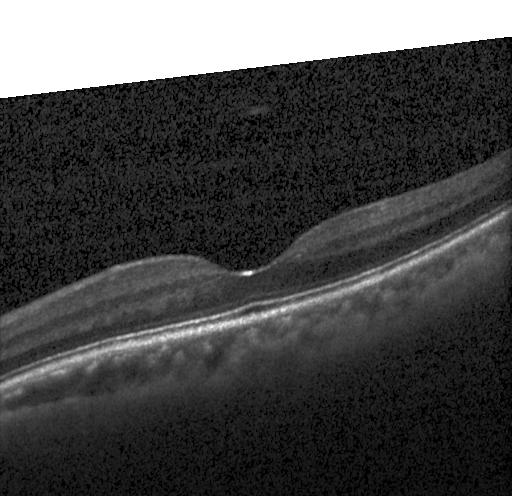
OCT B-scan — The scan shows no choroidal neovascularization, no diabetic macular edema, and no drusen.